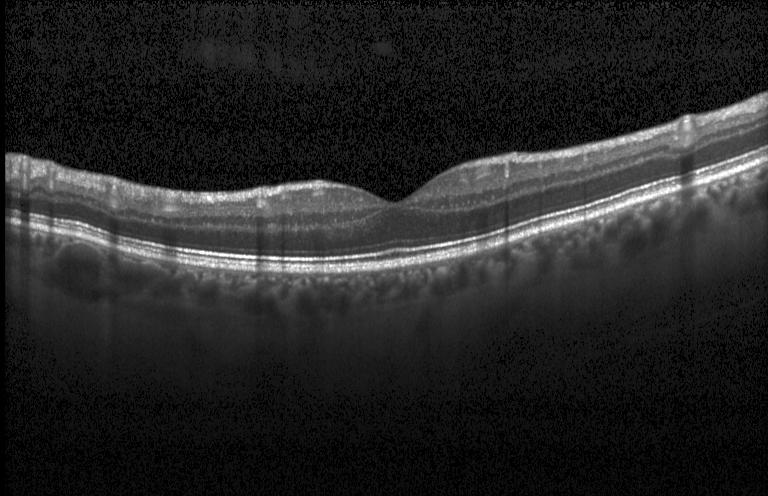
Heidelberg Spectralis OCT system; OCT B-scan — Assessment: no choroidal neovascularization, diabetic macular edema, or drusen.